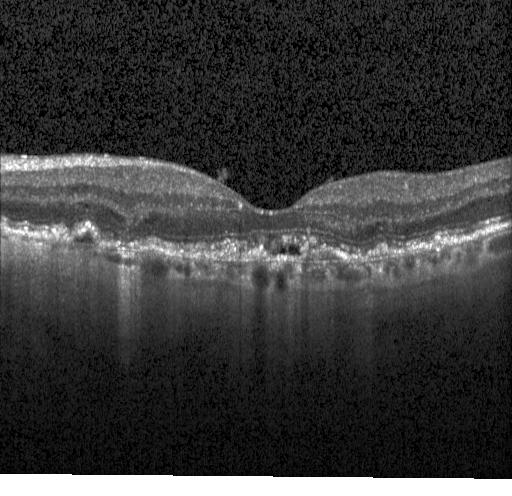

SD-OCT, OCT line scan.
Diagnosis: a choroidal neovascular membrane.